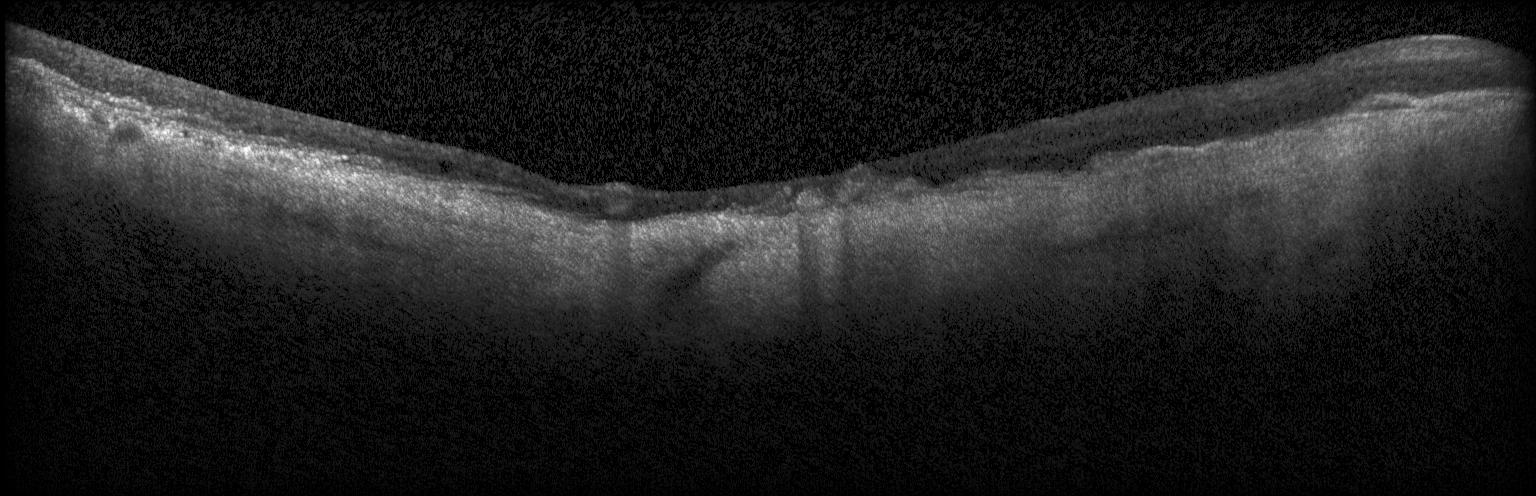 Macular OCT demonstrating choroidal neovascularization (CNV).